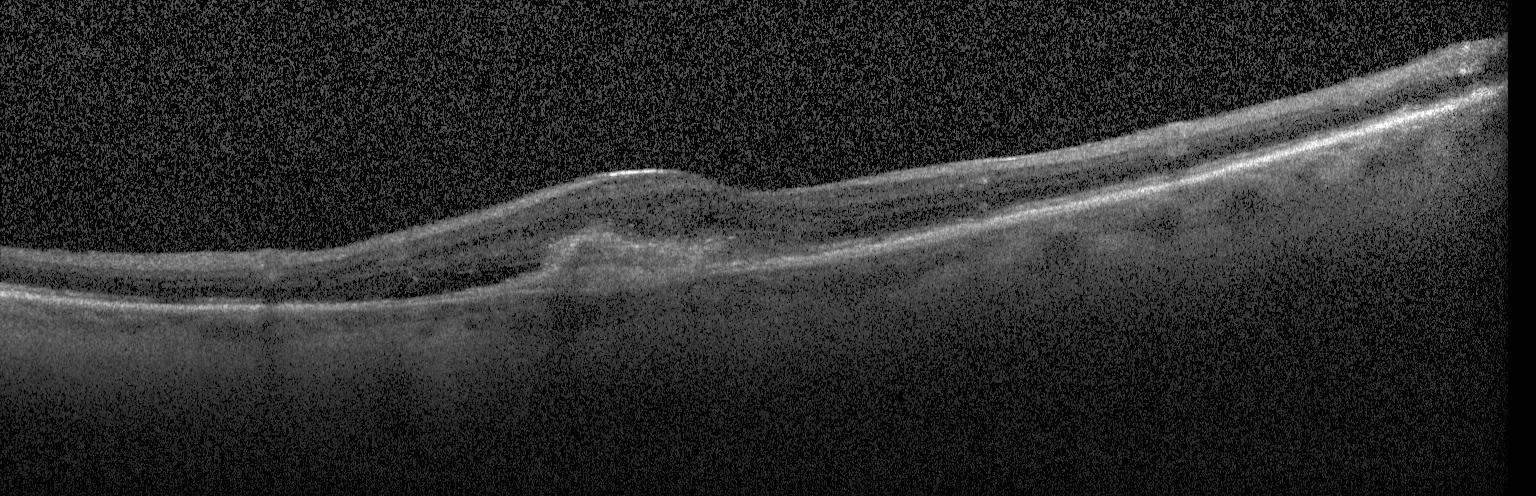

Retinal OCT B-scan. Horizontal scan through the fovea.
Choroidal neovascularization.